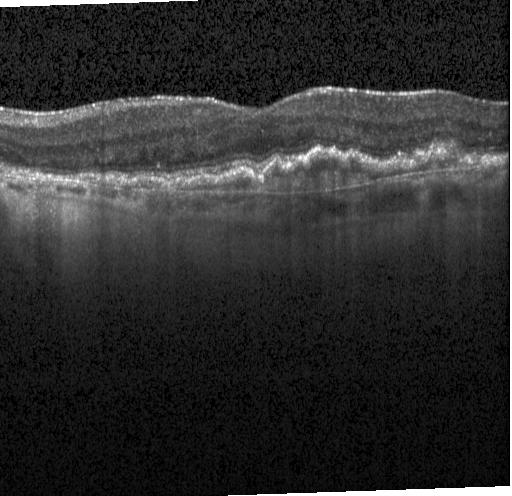

Impression: choroidal neovascularization (CNV).